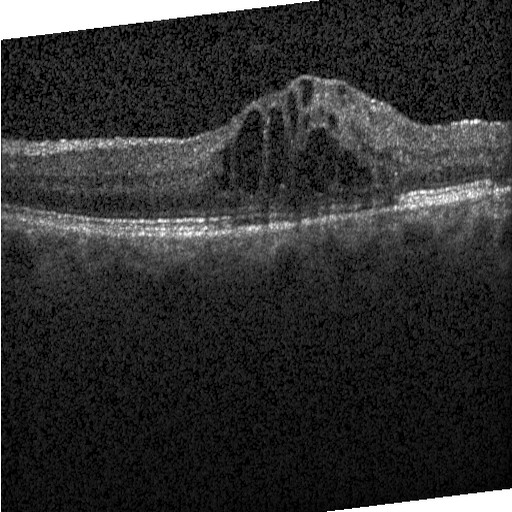 OCT scan showing DME.